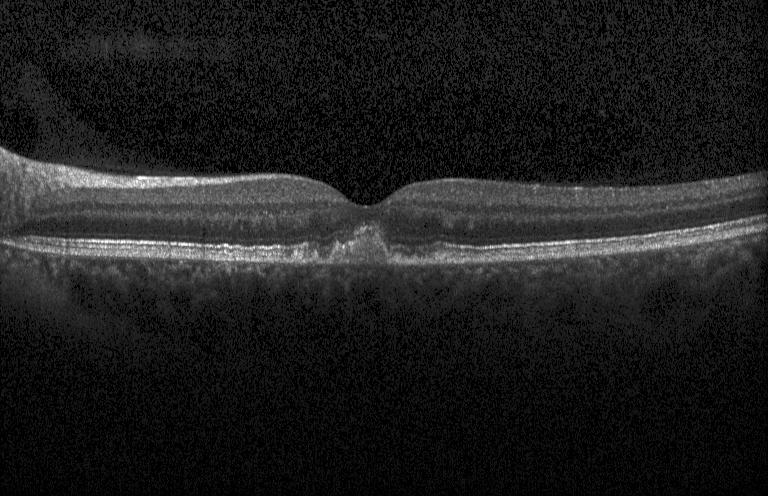
SD-OCT. Optical coherence tomography scan. The scan shows multiple drusen.